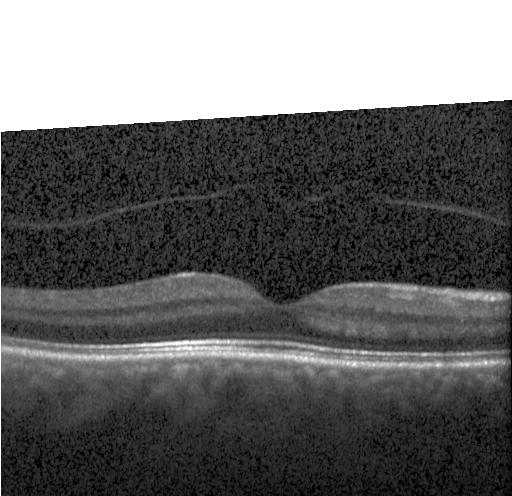
Spectral-domain OCT B-scan: no choroidal neovascularization, diabetic macular edema, or drusen.